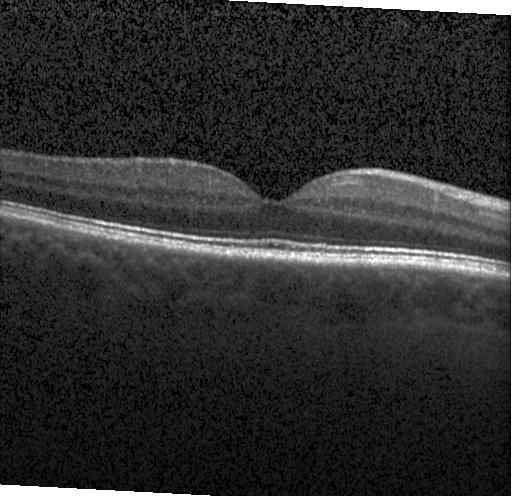 This B-scan demonstrates no CNV, DME, or drusen.